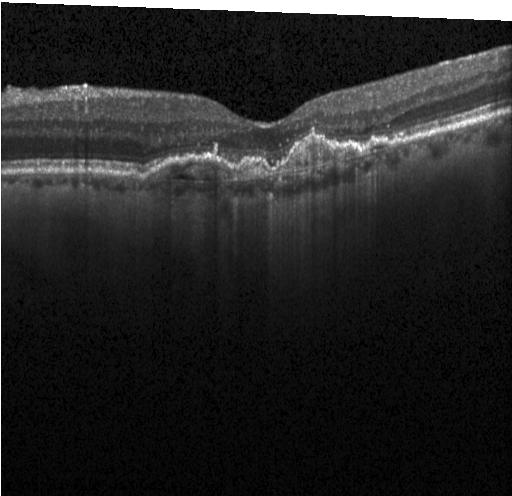
Optical coherence tomography B-scan; SD-OCT — Finding: choroidal neovascularization.